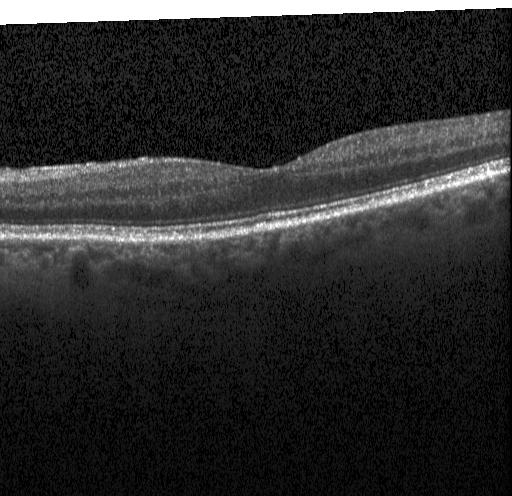 This B-scan demonstrates no evidence of choroidal neovascularization, diabetic macular edema, or drusen.